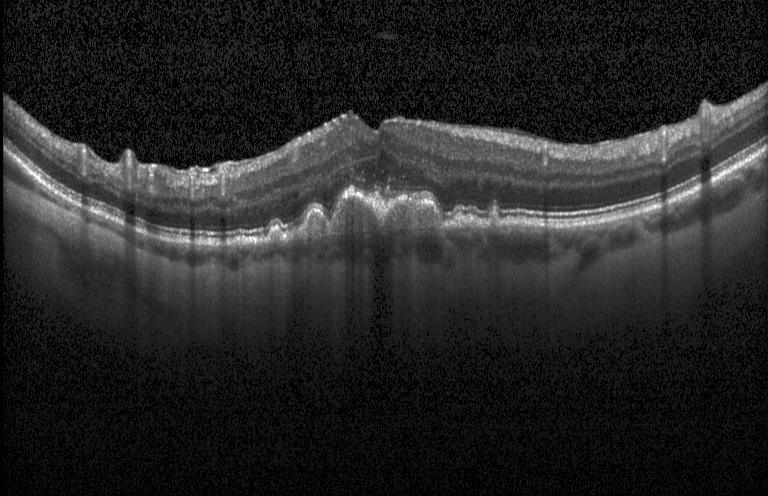

Finding: sub-RPE drusenoid deposits.